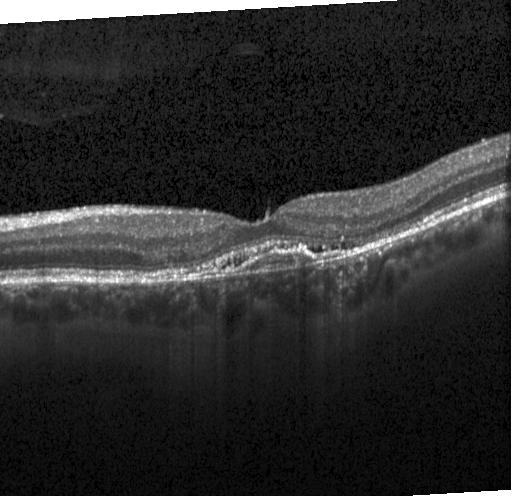 Optical coherence tomography B-scan.
Assessment: choroidal neovascularization.